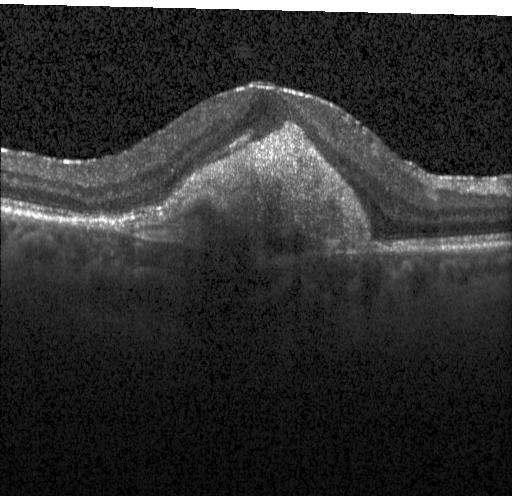 Spectral-domain OCT · Heidelberg Spectralis · retinal OCT cross-section — A choroidal neovascular membrane.